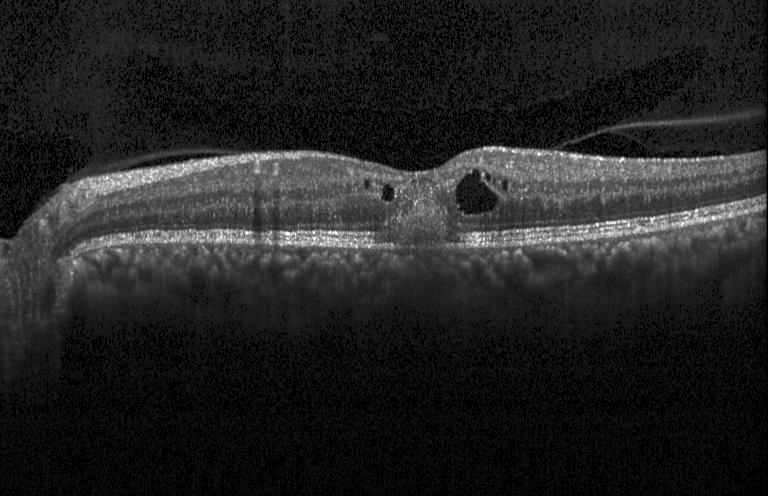

Impression: CNV.